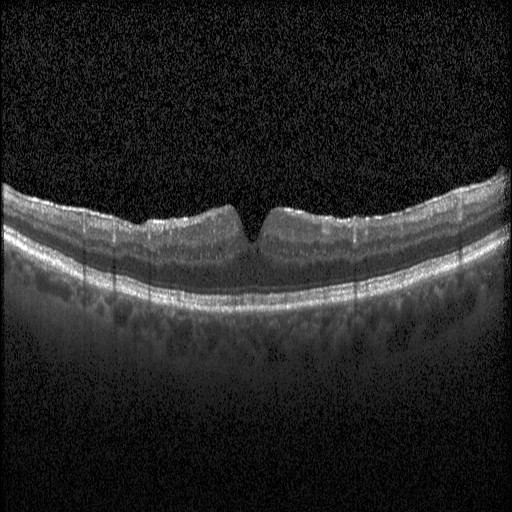 Macular scan · retinal OCT cross-section
Macular OCT: DME.